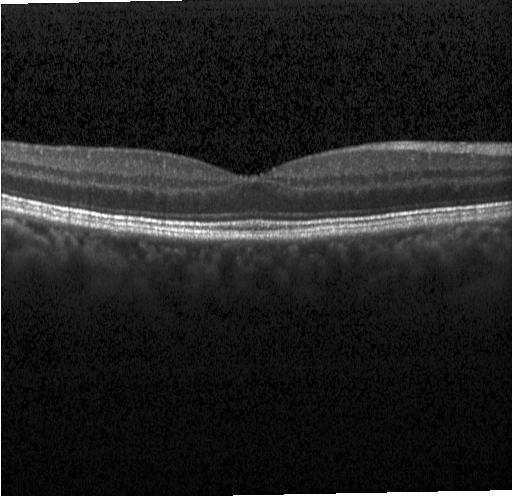
OCT finding: no evidence of CNV, DME, or drusen.